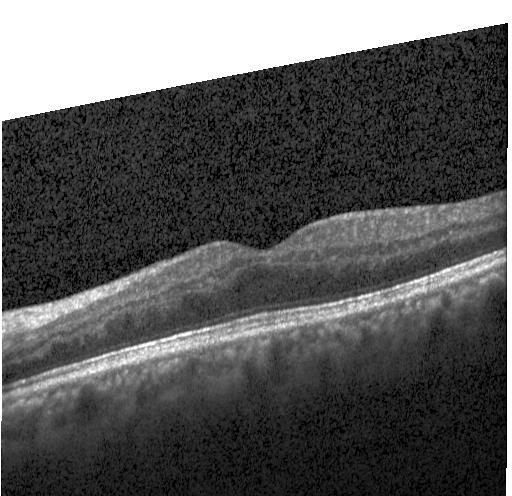

Fovea-centered · spectral-domain OCT · acquired on a Heidelberg Spectralis · OCT line scan.
Impression: no evidence of CNV, DME, or drusen.